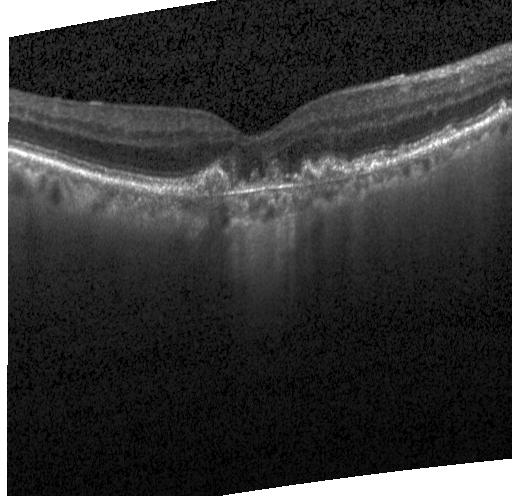
Retinal OCT B-scan, SD-OCT, Heidelberg Spectralis — The scan shows CNV.